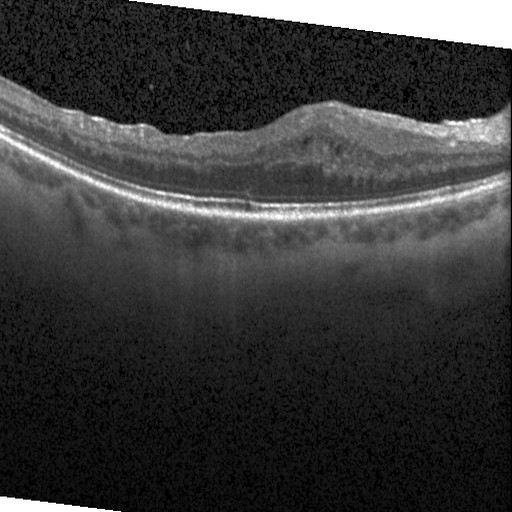

OCT line scan — This B-scan demonstrates DME.